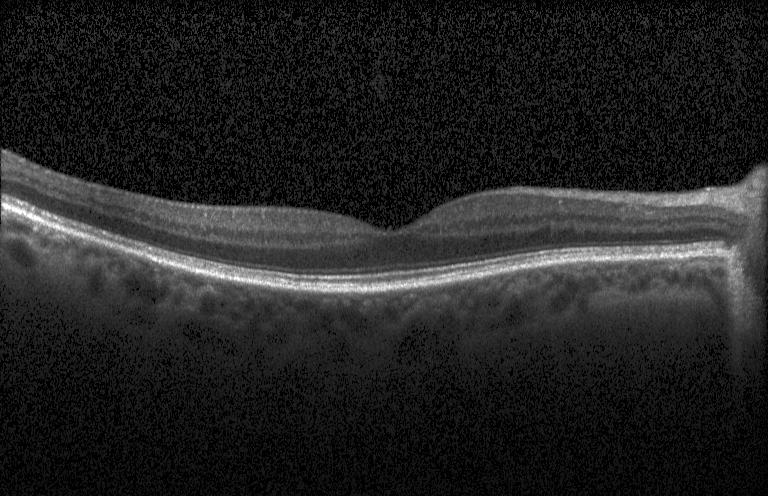 Macular scan · spectral-domain optical coherence tomography · OCT B-scan — Impression: no evidence of choroidal neovascularization, diabetic macular edema, or drusen.